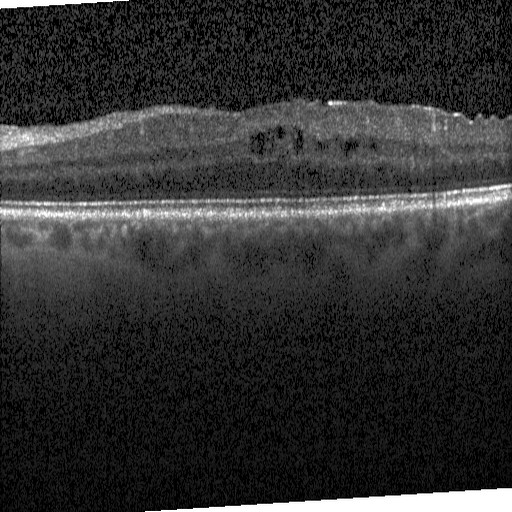

Impression: diabetic macular edema (DME).